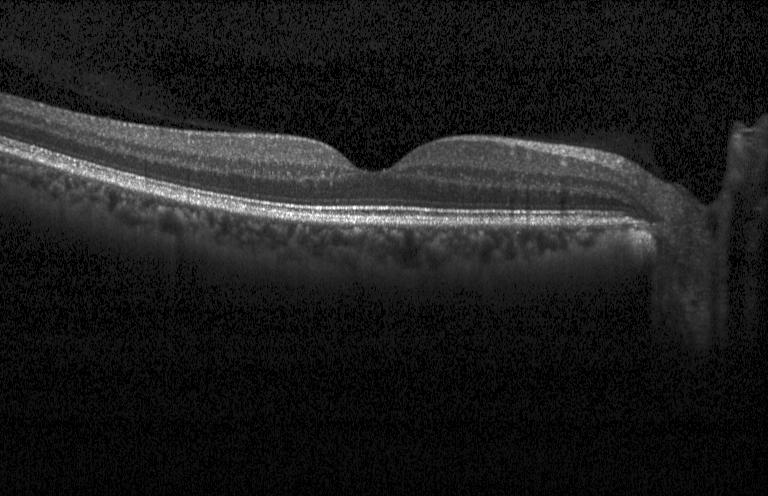

Finding: no CNV, DME, or drusen.